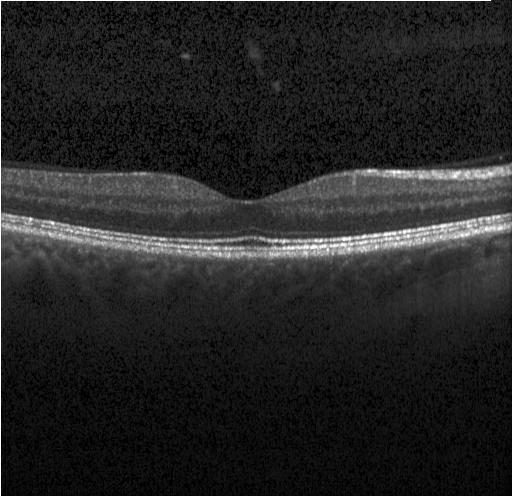 Retinal OCT B-scan.
No choroidal neovascularization, no diabetic macular edema, and no drusen.